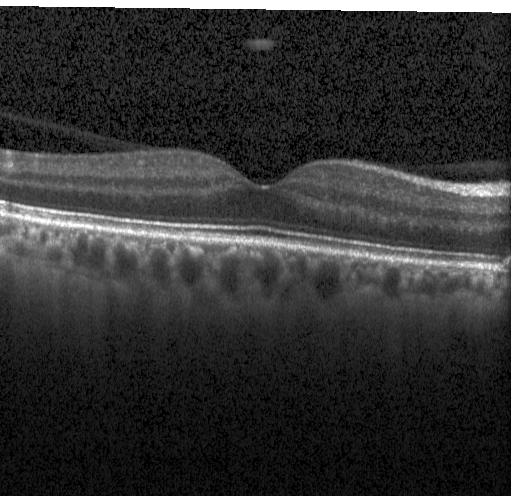 The scan shows no choroidal neovascularization, diabetic macular edema, or drusen.